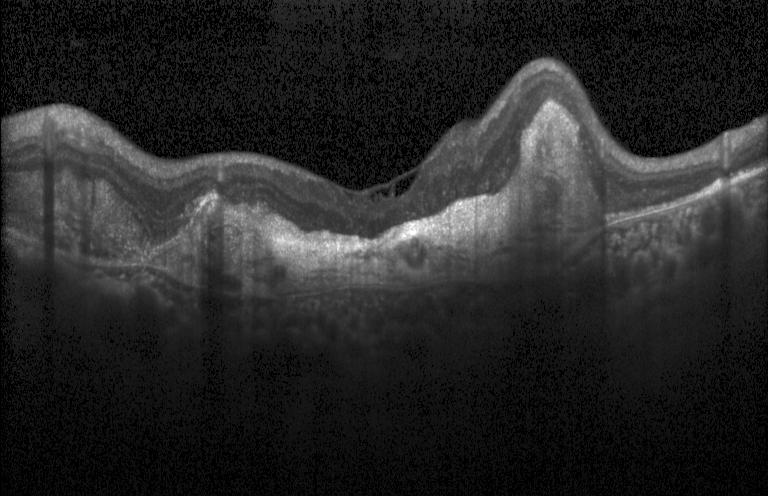
OCT line scan. Spectral-domain OCT — CNV.